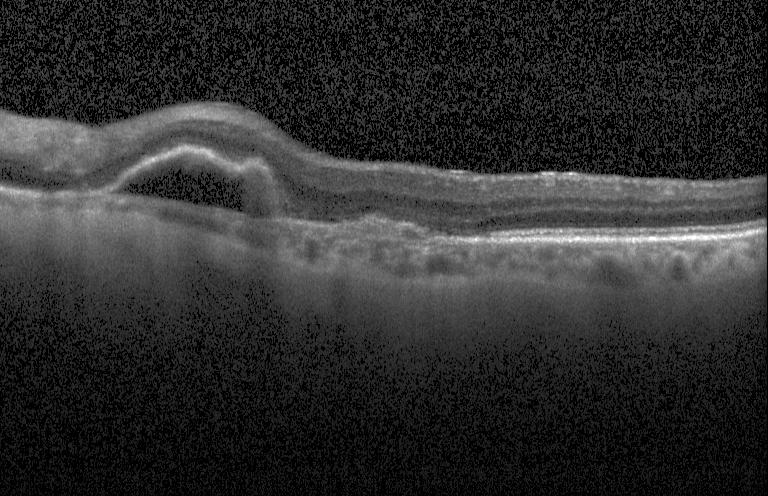
Spectral-domain OCT, horizontal scan through the fovea, Heidelberg Spectralis, OCT line scan — Assessment: a choroidal neovascular membrane.